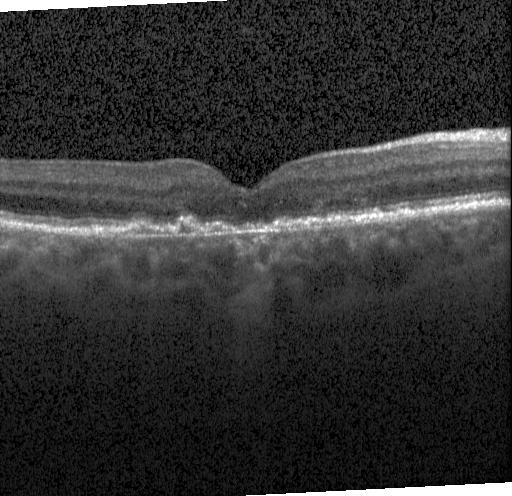 Acquired on a Heidelberg Spectralis, OCT B-scan.
Assessment: a choroidal neovascular membrane.